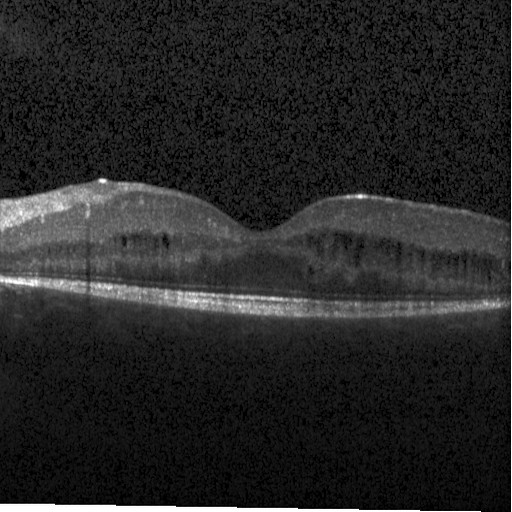
Instrument: Heidelberg Spectralis · SD-OCT · OCT B-scan — Macular OCT: DME.